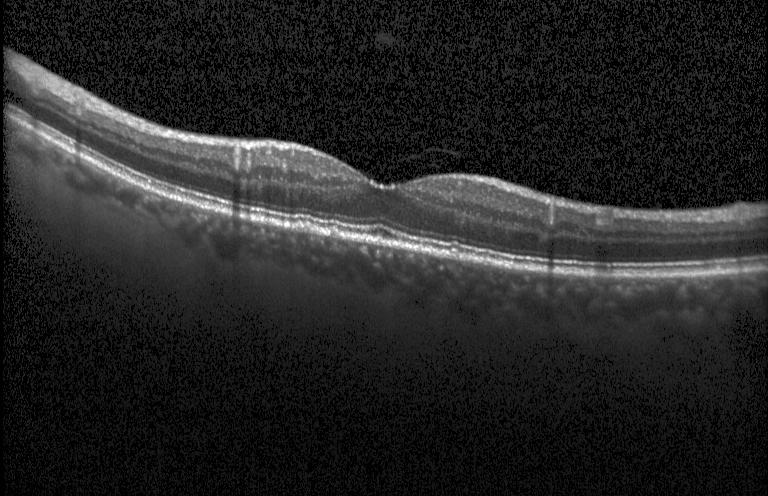
Optical coherence tomography scan.
Impression: drusen.